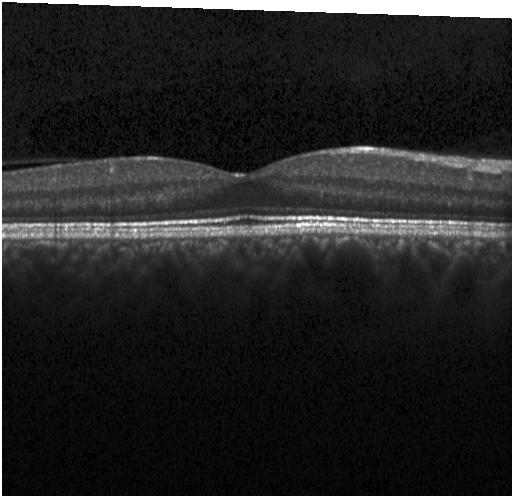

The scan shows no choroidal neovascularization, diabetic macular edema, or drusen.